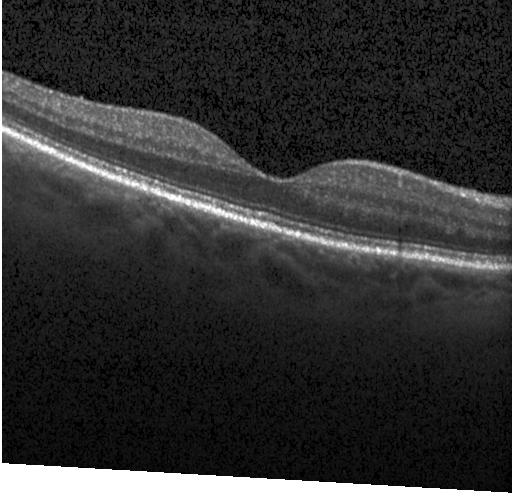

Dx: no choroidal neovascularization, diabetic macular edema, or drusen.